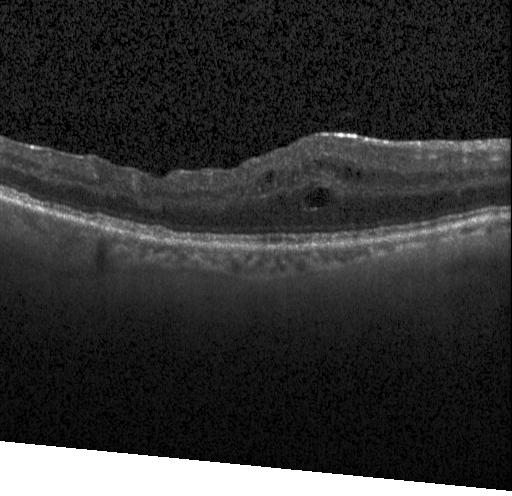

Optical coherence tomography B-scan. Centered on the fovea — Macular OCT: DME.